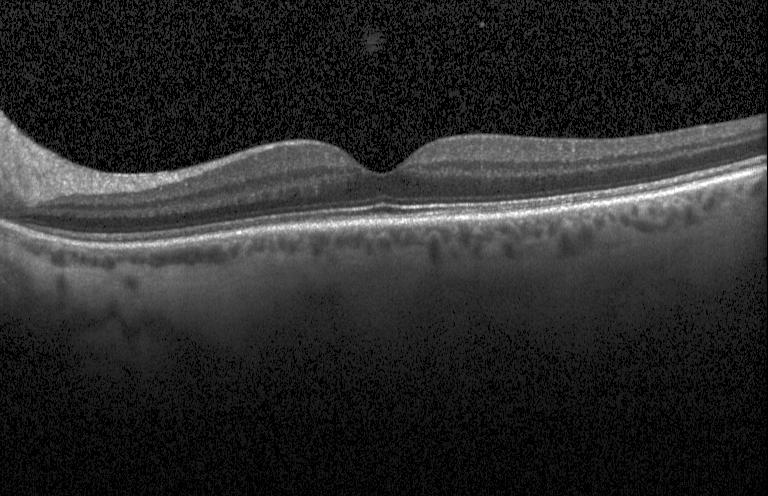

Retinal OCT cross-section showing no CNV, no DME, and no drusen.